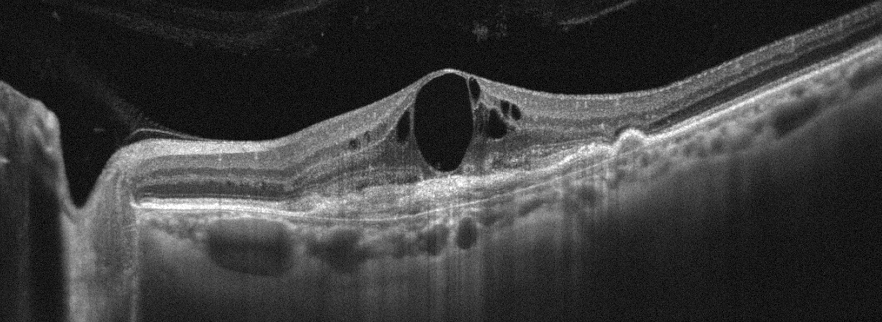 OS; retinal OCT B-scan. The scan shows AMD.